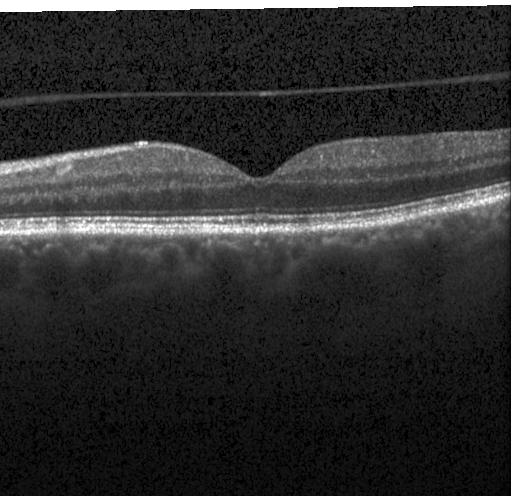

Spectral-domain optical coherence tomography. OCT B-scan — Impression: neither CNV, DME, nor drusen.